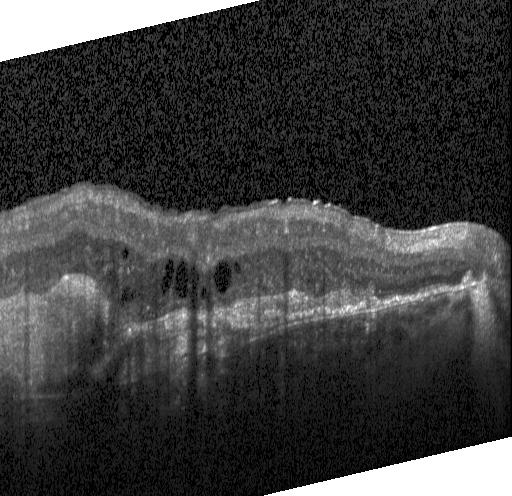
Finding: choroidal neovascularization.